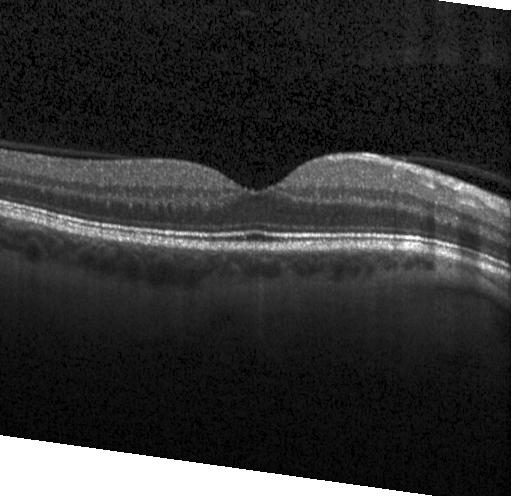 SD-OCT · OCT B-scan · Heidelberg Spectralis OCT system.
Finding: no choroidal neovascularization, diabetic macular edema, or drusen.